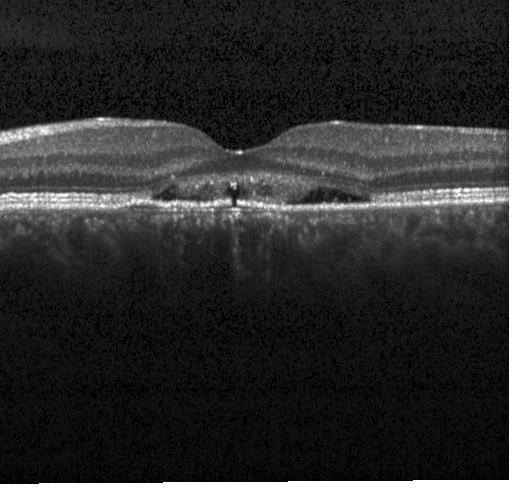
OCT line scan — The scan shows a choroidal neovascular membrane.